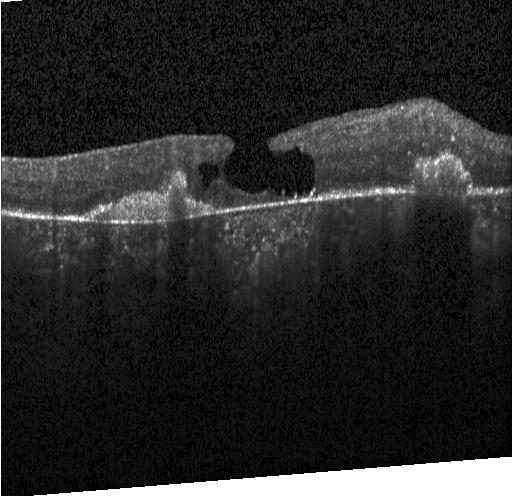 Finding: choroidal neovascularization (CNV).